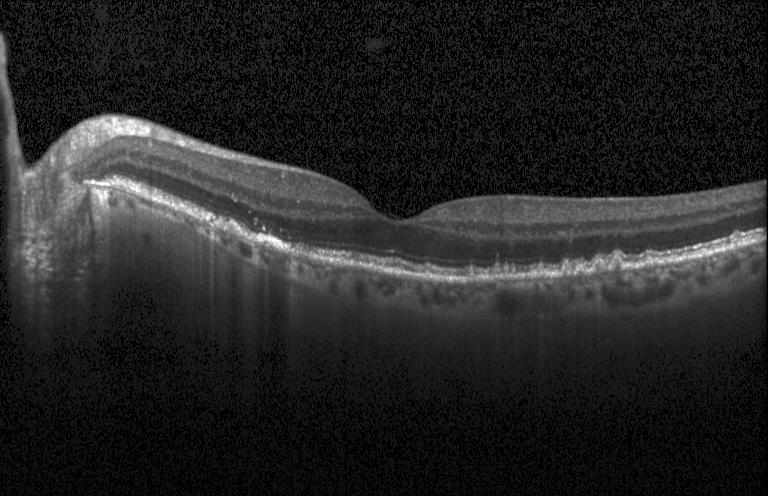
Drusen.